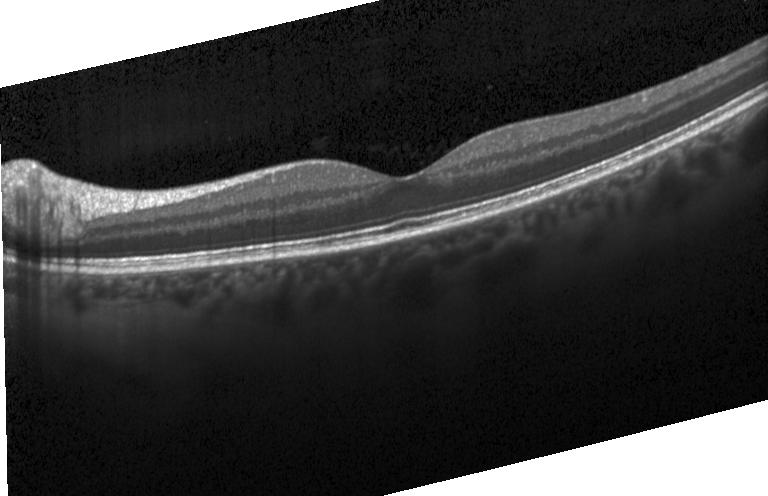
Fovea-centered; OCT line scan. Macular OCT: no choroidal neovascularization, no diabetic macular edema, and no drusen.